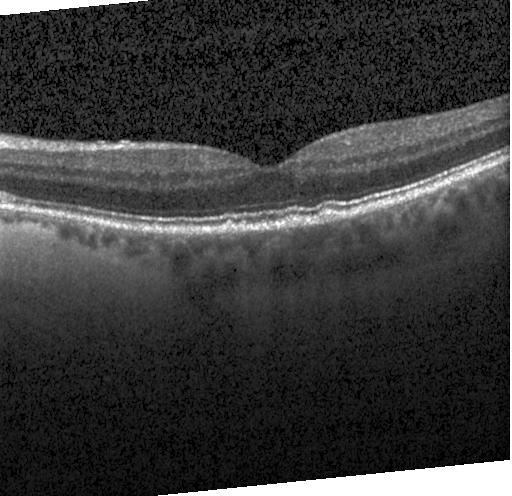

Retinal OCT cross-section
Finding: sub-RPE drusenoid deposits.